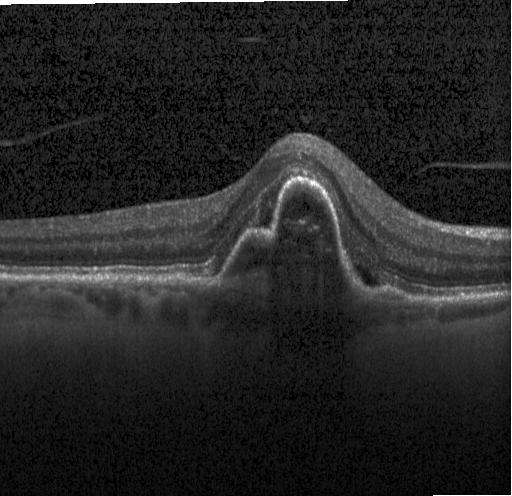
Optical coherence tomography scan — CNV.